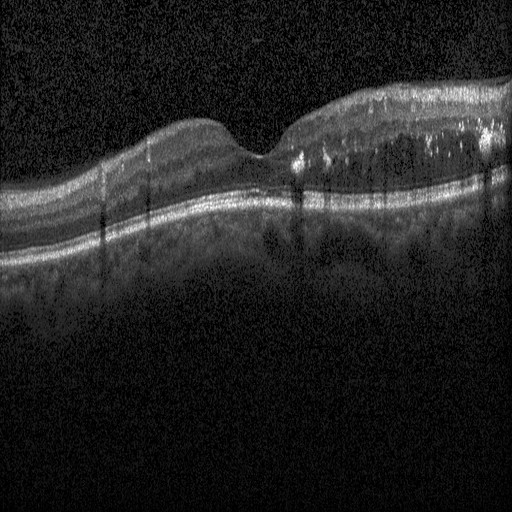
Acquired on a Heidelberg Spectralis; SD-OCT; through the macula; retinal OCT B-scan
Finding: diabetic macular edema.